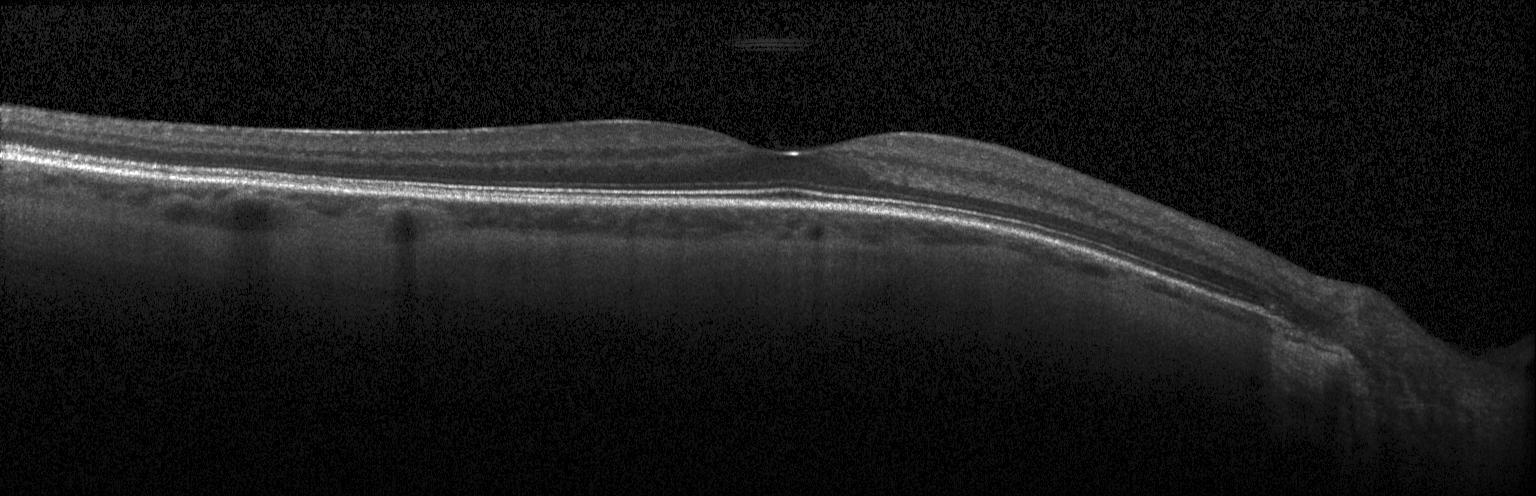 Retinal OCT cross-section showing no choroidal neovascularization, diabetic macular edema, or drusen.